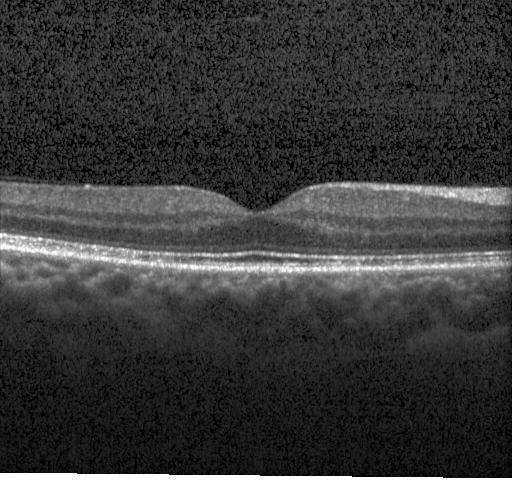
Impression: no evidence of choroidal neovascularization, diabetic macular edema, or drusen.